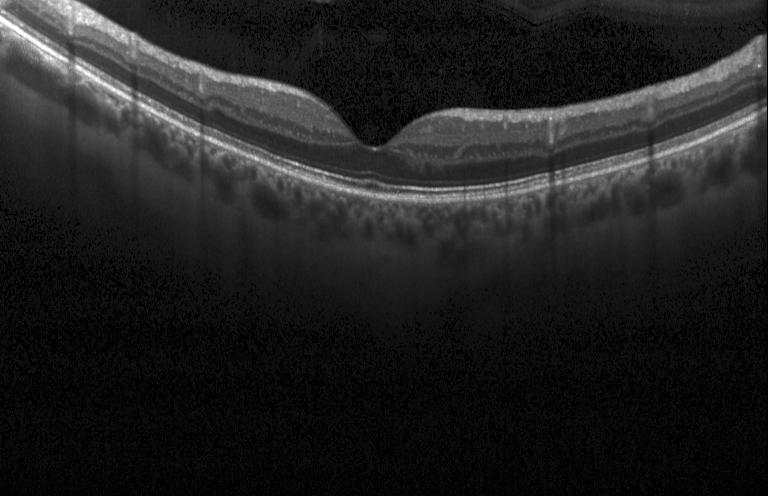

Impression: no choroidal neovascularization, no diabetic macular edema, and no drusen.